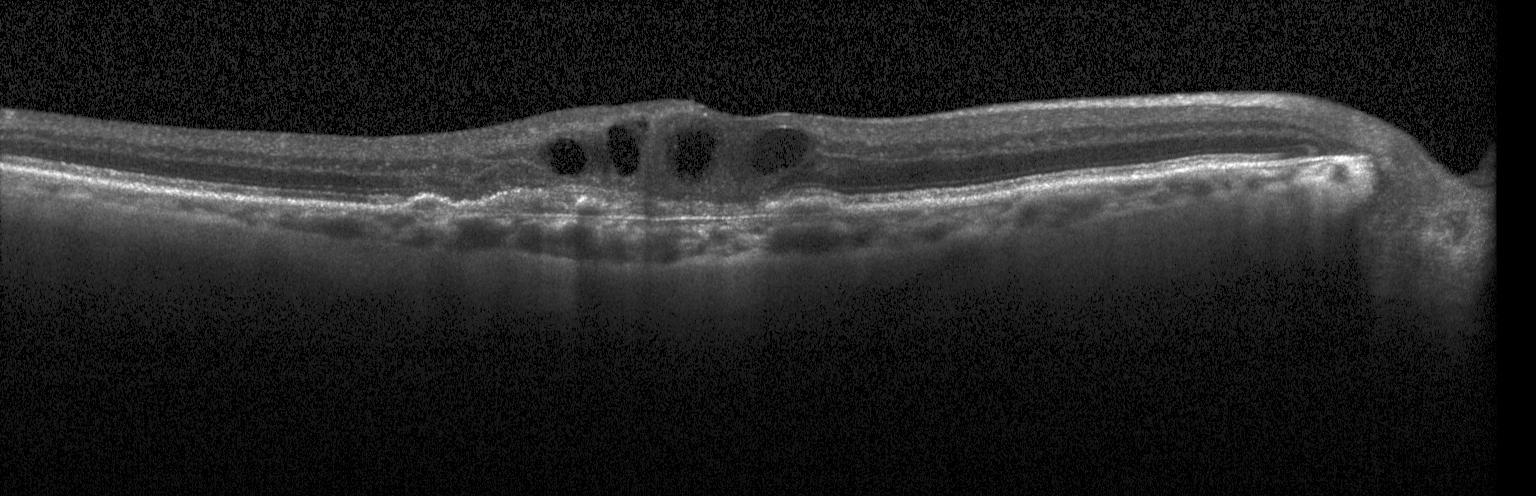
SD-OCT · horizontal scan through the fovea · OCT line scan.
The scan shows choroidal neovascularization.